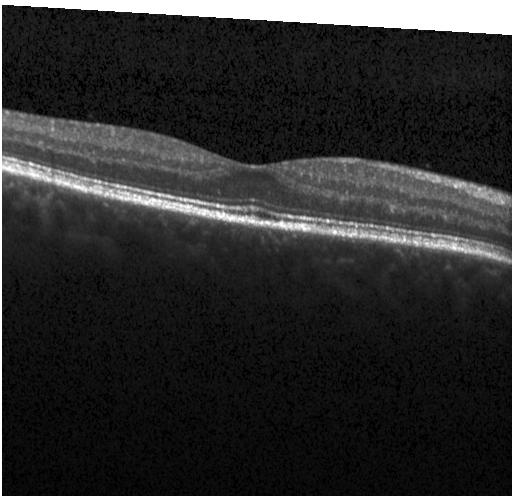

Spectral-domain OCT B-scan: neither CNV, DME, nor drusen.